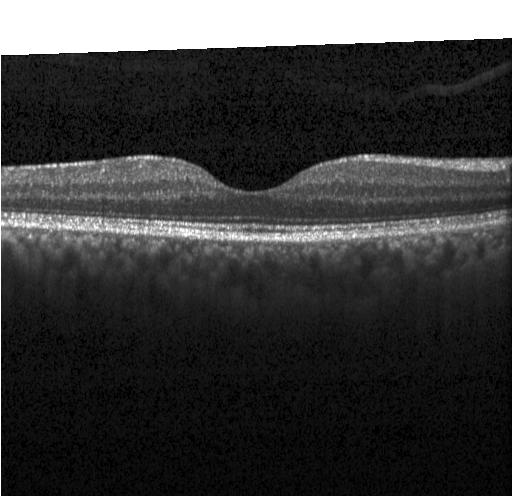

Spectral-domain OCT, OCT B-scan, macular scan, Heidelberg Spectralis. Macular OCT: no evidence of choroidal neovascularization, diabetic macular edema, or drusen.